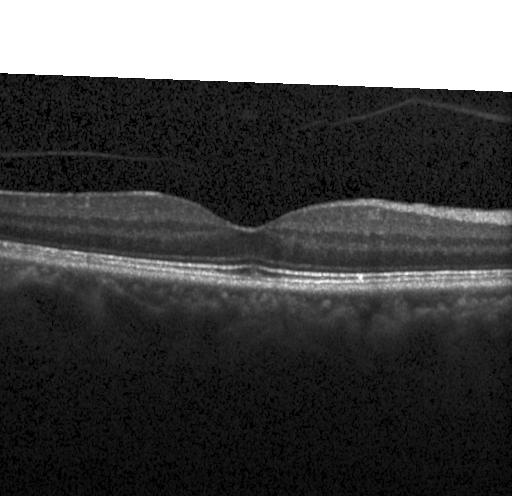
Spectral-domain OCT B-scan: neither CNV, DME, nor drusen.